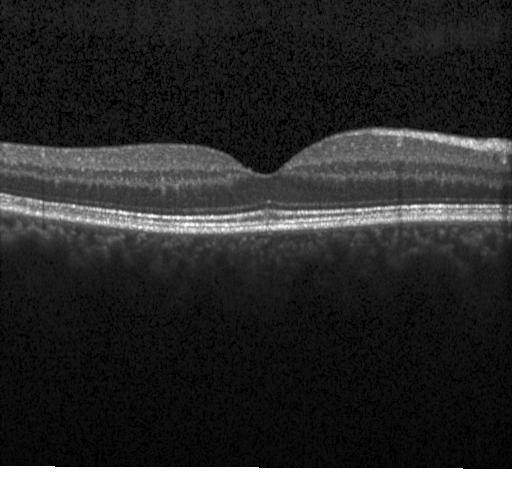
Horizontal scan through the fovea · spectral-domain optical coherence tomography · Heidelberg Spectralis OCT system · OCT line scan
Diagnosis: neither choroidal neovascularization, diabetic macular edema, nor drusen.